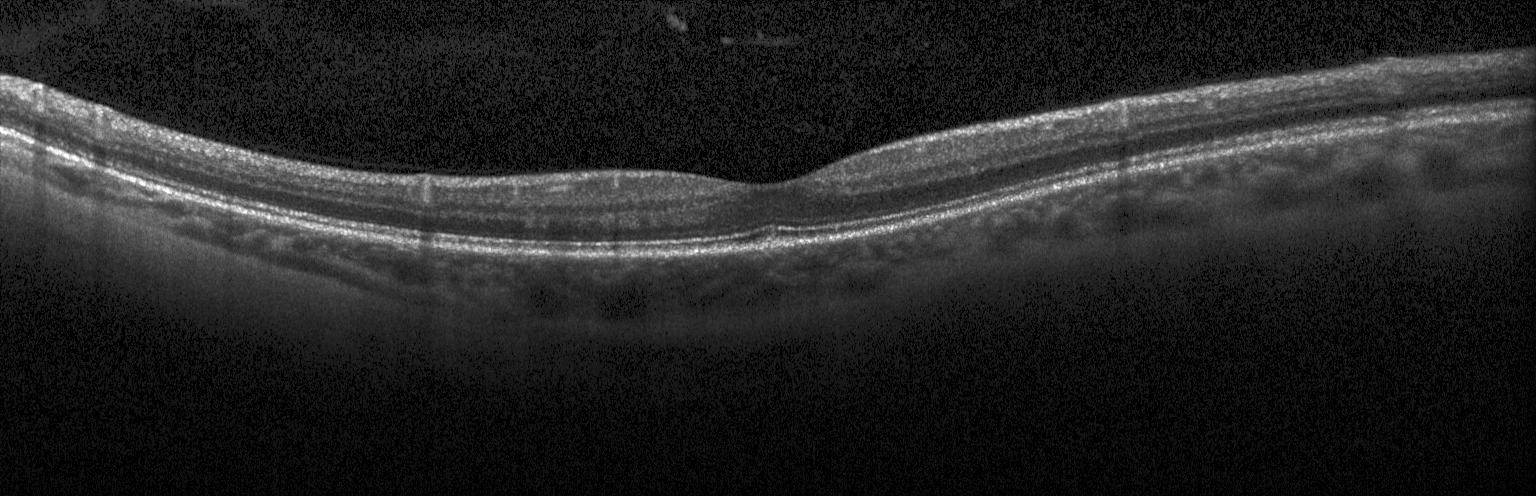

OCT B-scan showing no choroidal neovascularization, diabetic macular edema, or drusen.